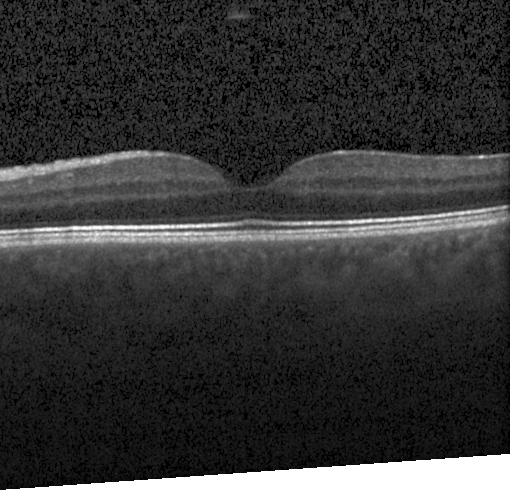

Finding: no evidence of choroidal neovascularization, diabetic macular edema, or drusen.